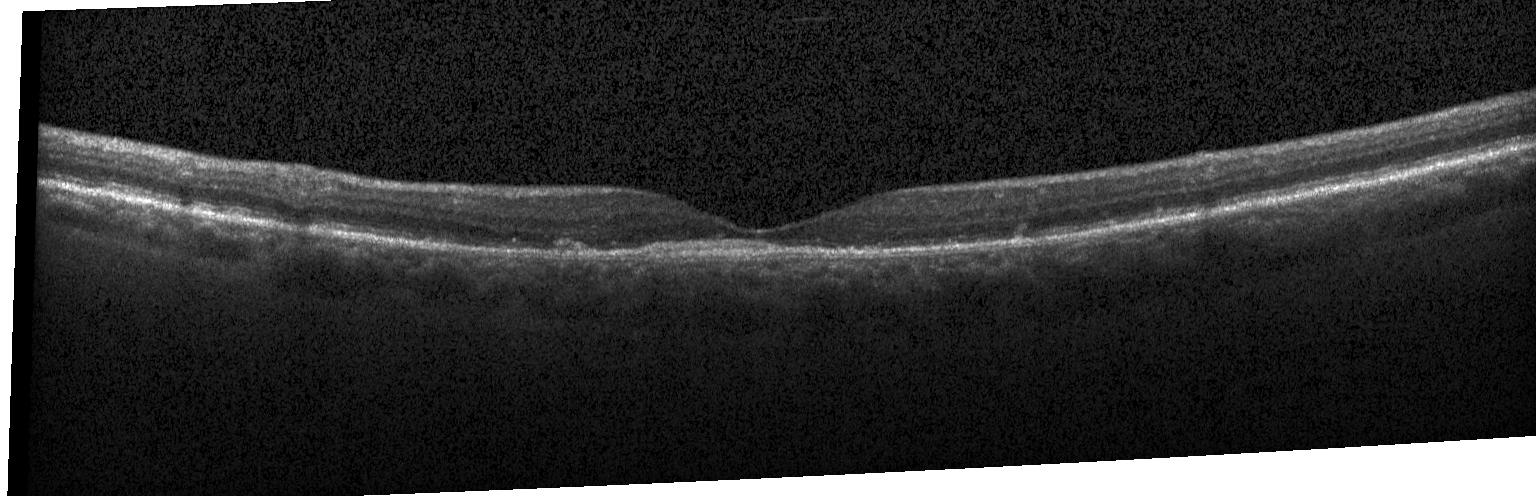
Diagnosis: a choroidal neovascular membrane.